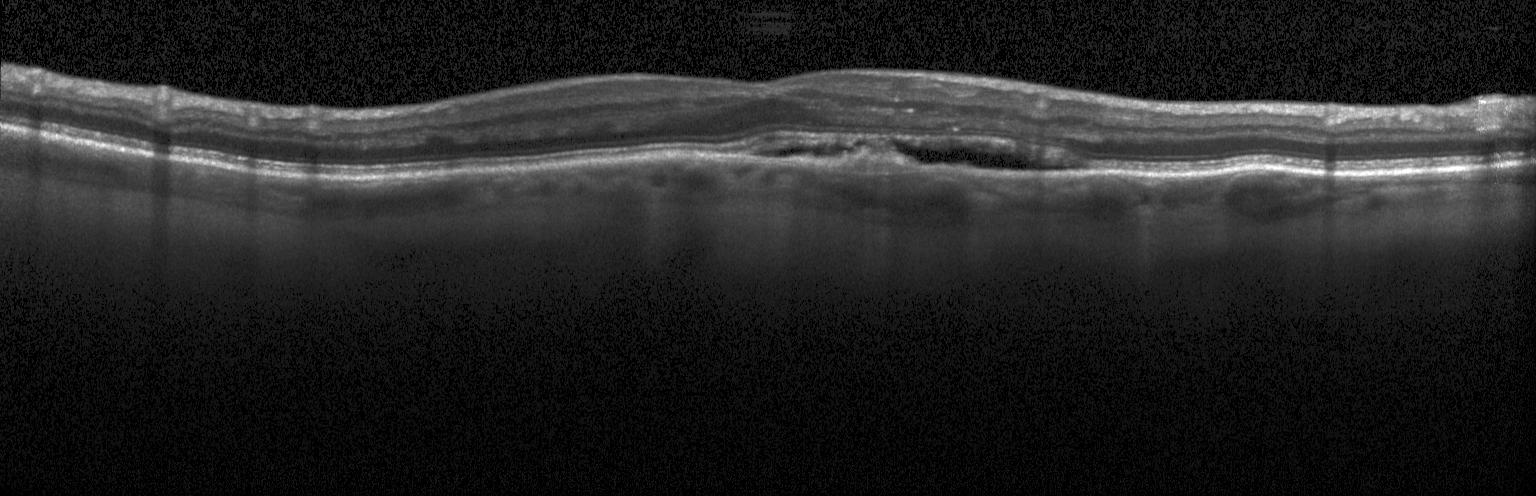
Macular OCT demonstrating a choroidal neovascular membrane.